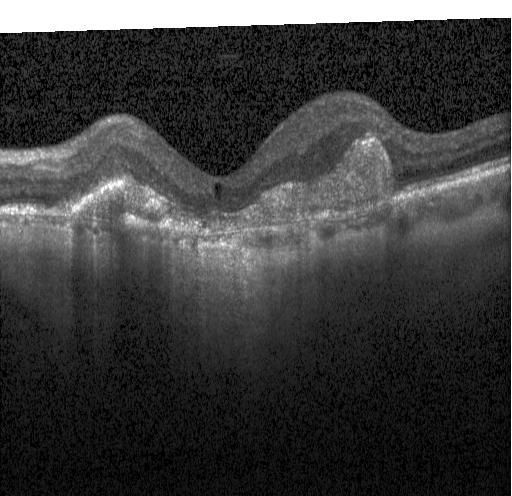
This B-scan demonstrates choroidal neovascularization.